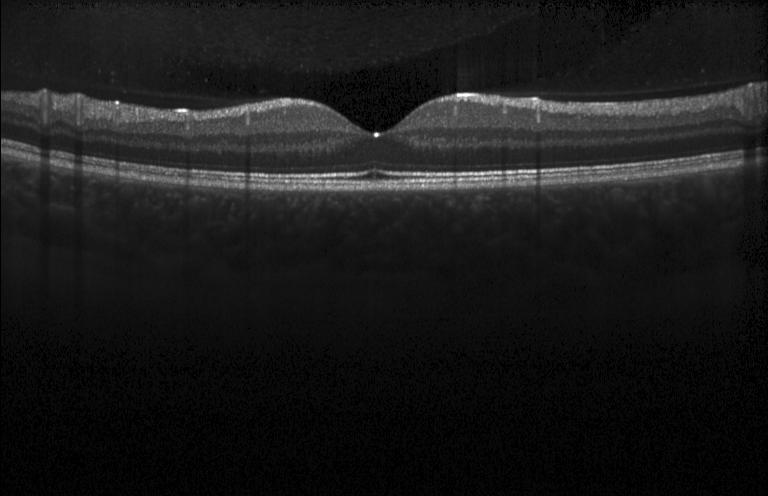 OCT B-scan showing no CNV, no DME, and no drusen.